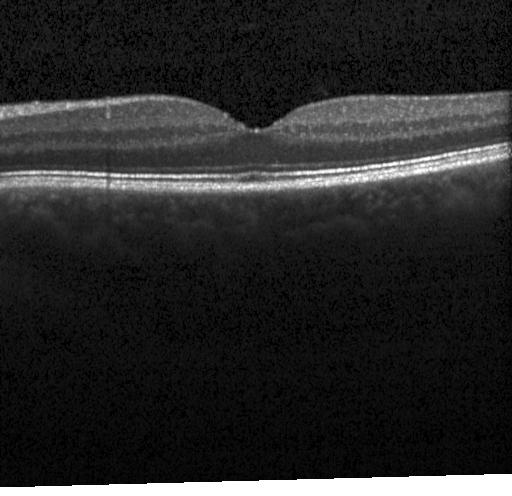
Dx: no CNV, DME, or drusen.